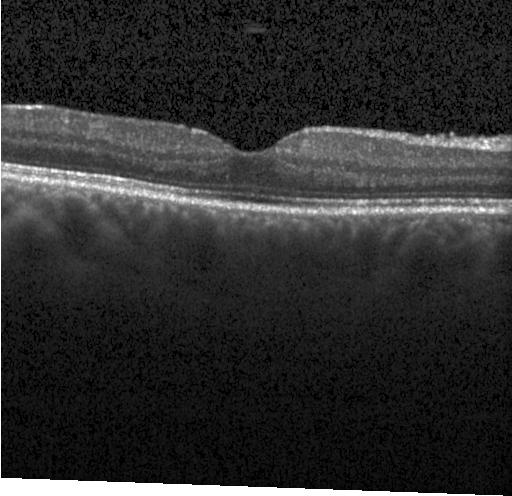

OCT scan showing no CNV, no DME, and no drusen.